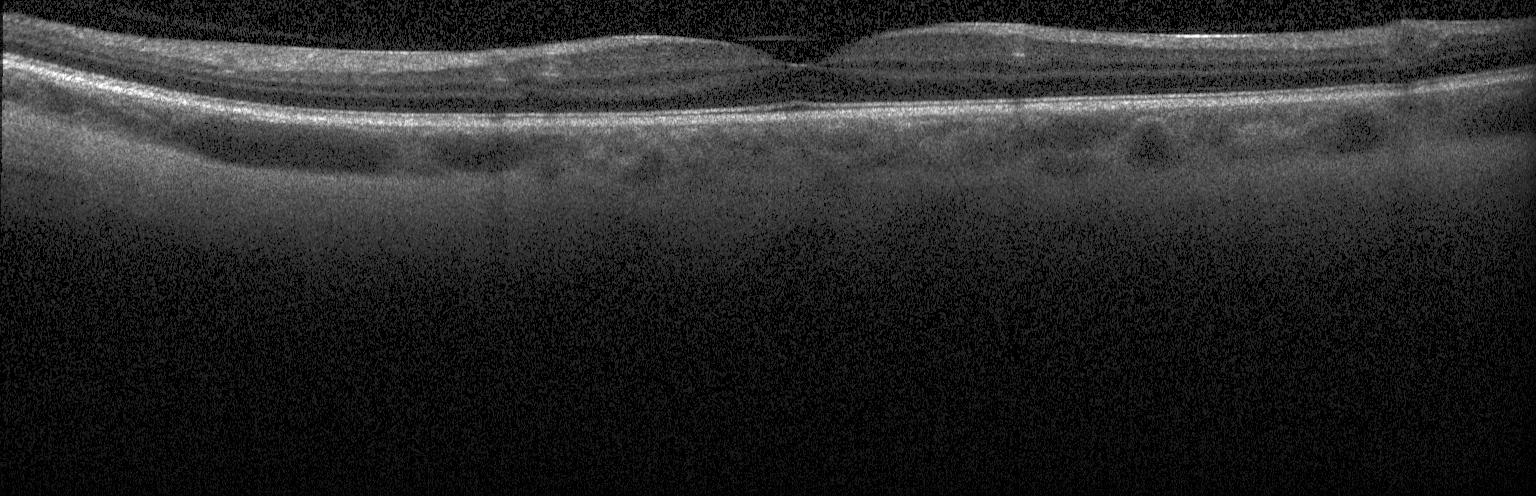 OCT finding: no choroidal neovascularization, diabetic macular edema, or drusen.